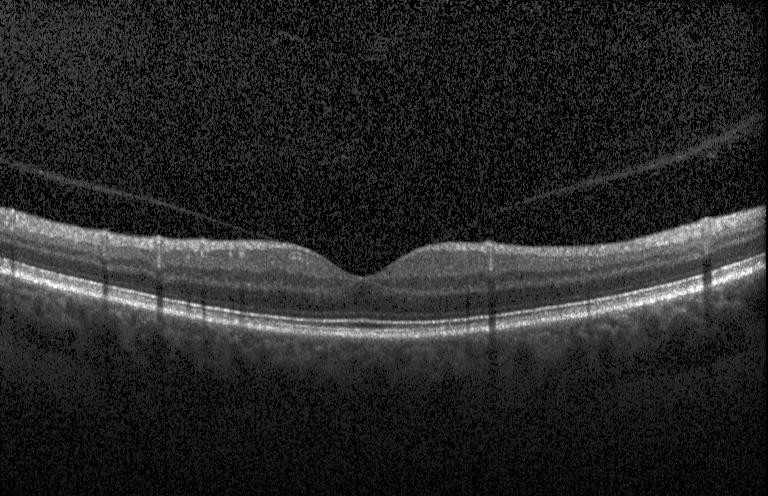
Heidelberg Spectralis OCT system · retinal OCT B-scan.
OCT finding: neither choroidal neovascularization, diabetic macular edema, nor drusen.